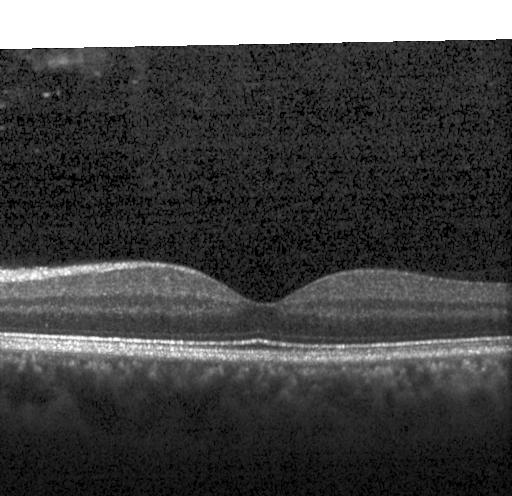

Macular scan · instrument: Heidelberg Spectralis · optical coherence tomography B-scan — Dx: no evidence of choroidal neovascularization, diabetic macular edema, or drusen.